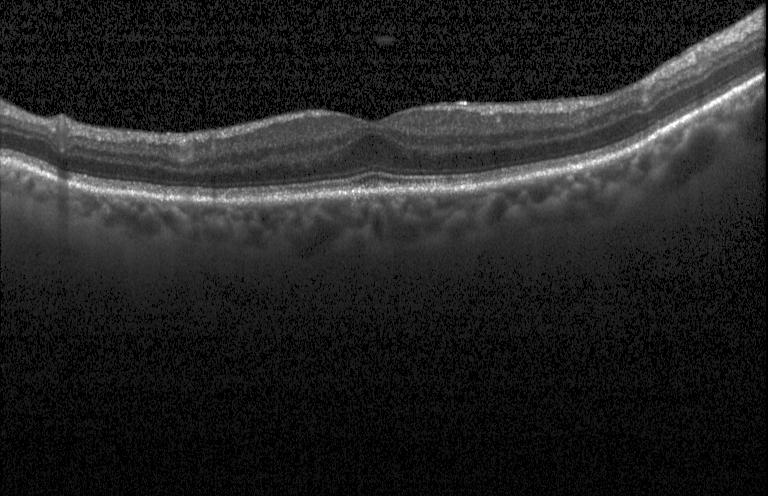 Heidelberg Spectralis; OCT B-scan.
Impression: neither choroidal neovascularization, diabetic macular edema, nor drusen.